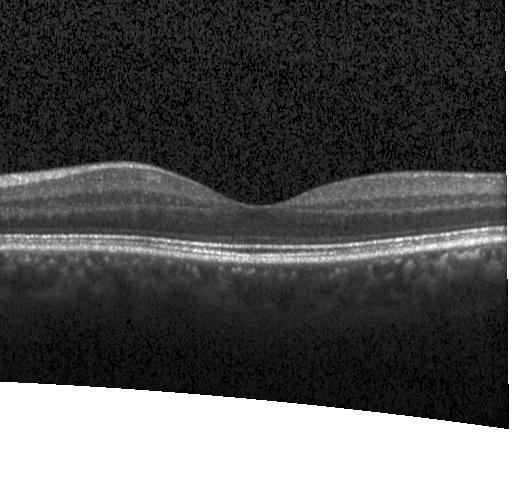

Retinal OCT B-scan. Heidelberg Spectralis OCT system. Spectral-domain OCT.
No CNV, DME, or drusen.